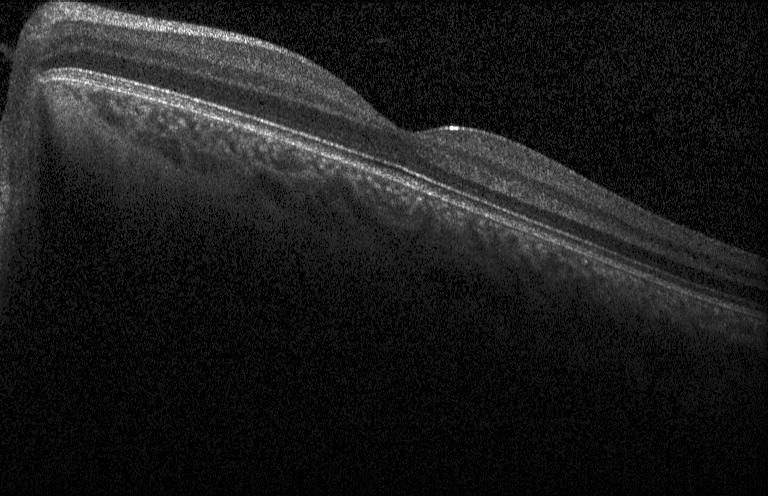

Finding: no CNV, DME, or drusen.